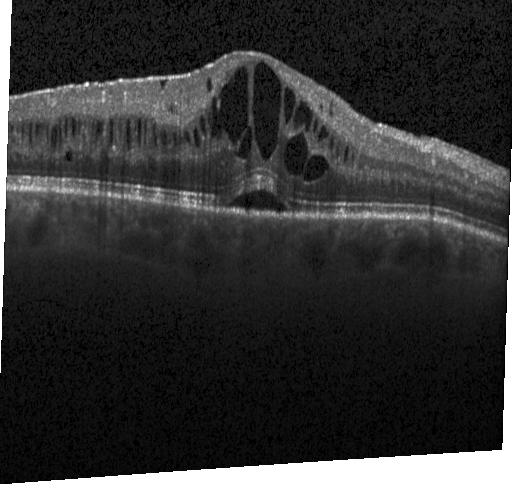

Macular OCT: diabetic macular edema.